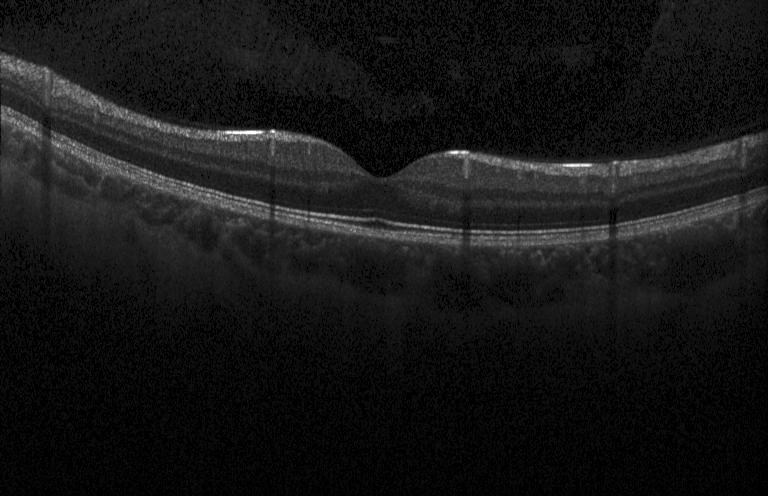 Optical coherence tomography B-scan, spectral-domain optical coherence tomography. This B-scan demonstrates no choroidal neovascularization, diabetic macular edema, or drusen.